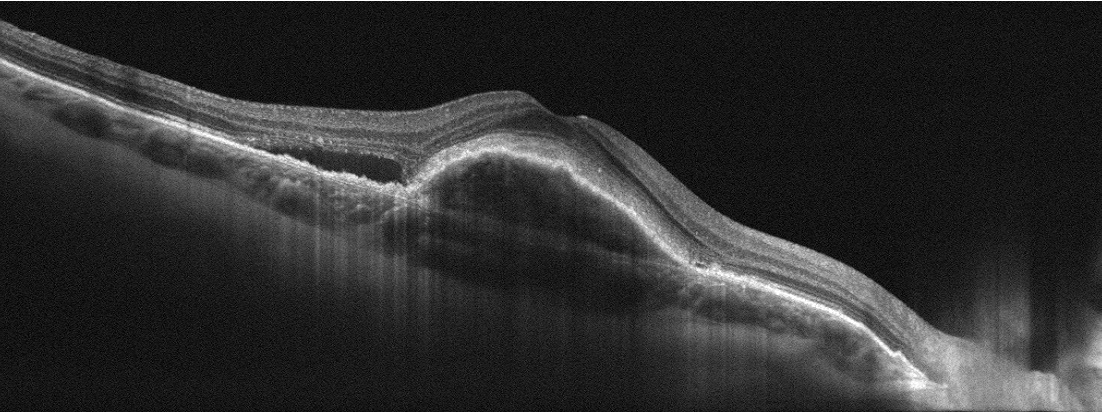
Optical coherence tomography scan · macular scan · Optovue Avanti RTVue XR. Finding: age-related macular degeneration (AMD).